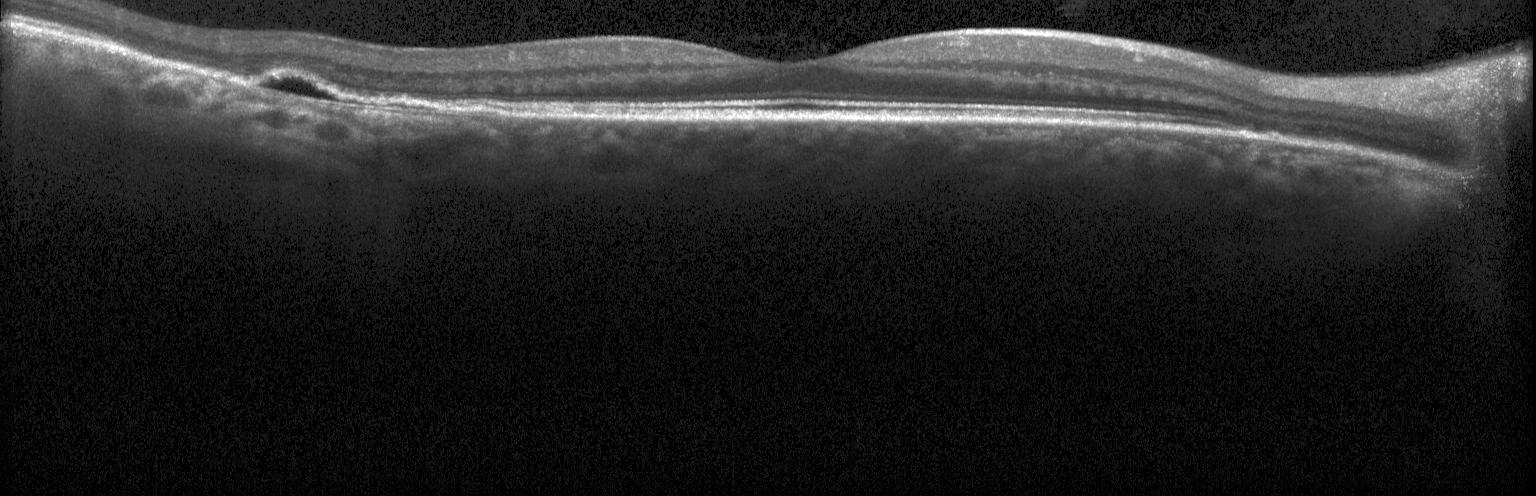

OCT B-scan.
Impression: a choroidal neovascular membrane.